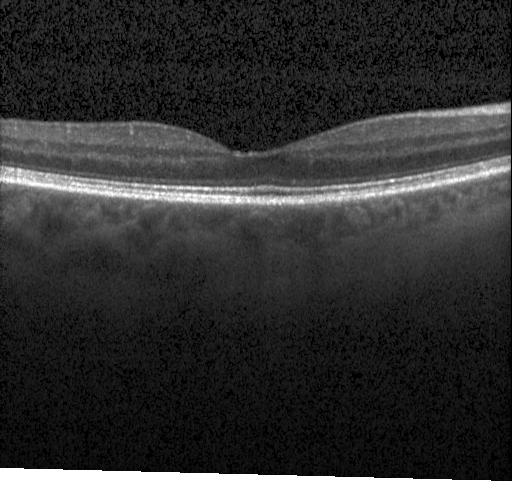
Optical coherence tomography B-scan; spectral-domain OCT; horizontal scan through the fovea; Heidelberg Spectralis OCT system — Neither choroidal neovascularization, diabetic macular edema, nor drusen.